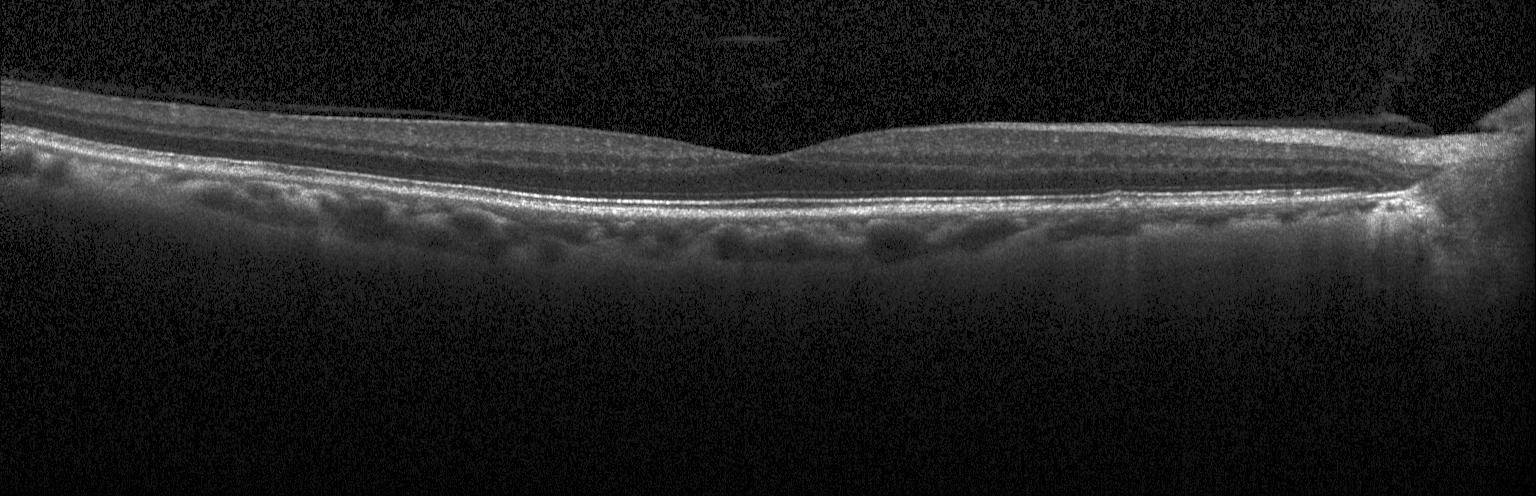 This B-scan demonstrates no evidence of CNV, DME, or drusen.